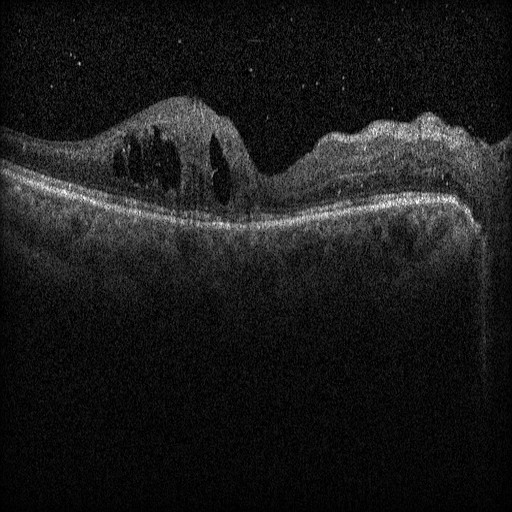
Macular OCT: diabetic macular edema.